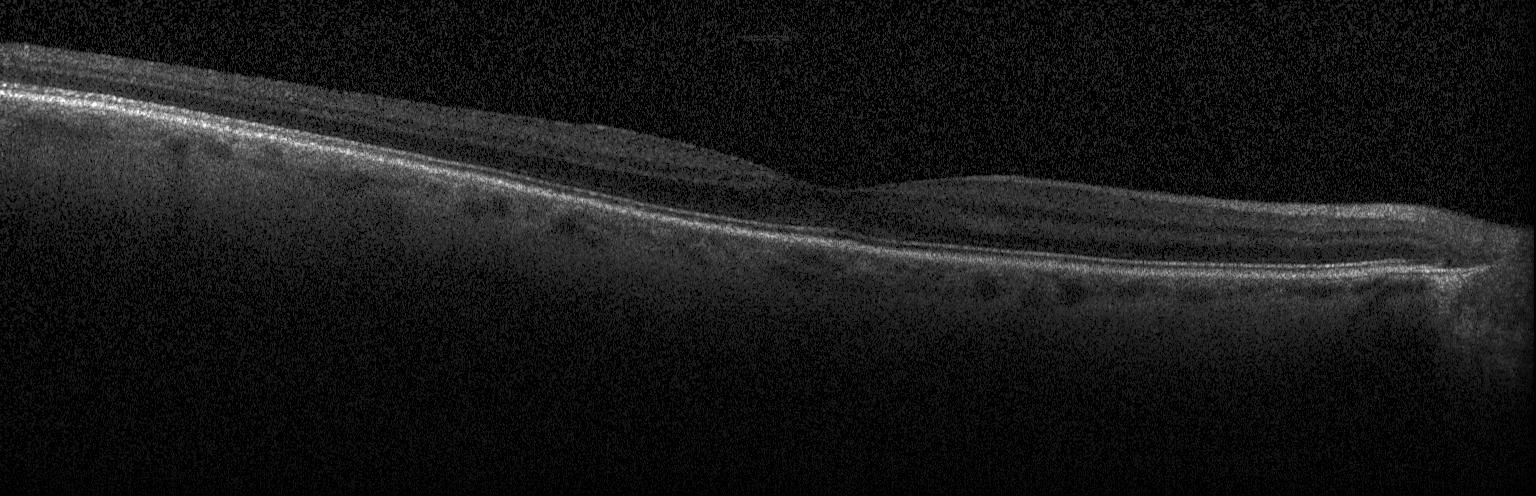 Macular scan. OCT B-scan. Assessment: neither choroidal neovascularization, diabetic macular edema, nor drusen.